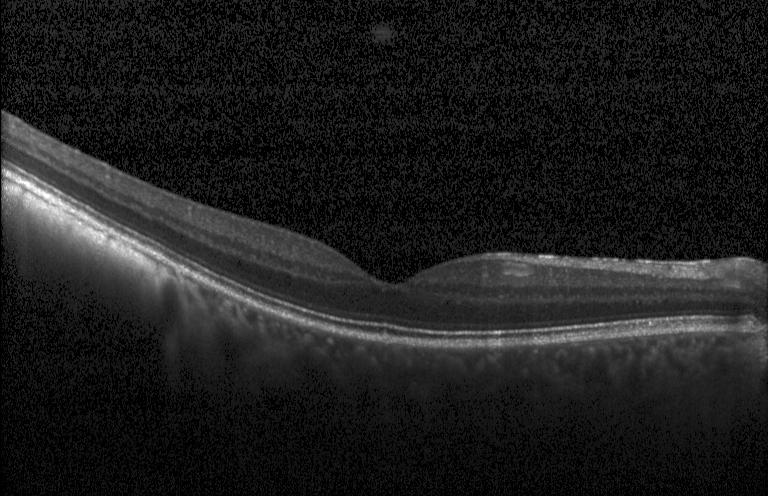
OCT line scan
Impression: sub-RPE drusenoid deposits.